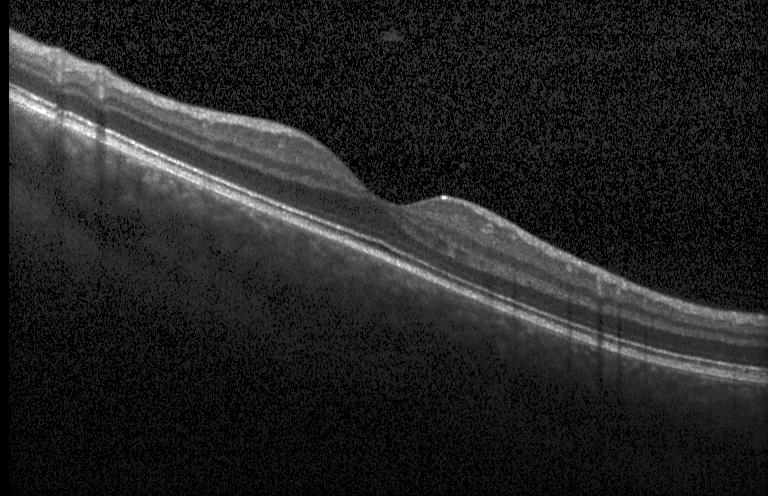
Horizontal scan through the fovea · retinal OCT B-scan · Heidelberg Spectralis · spectral-domain OCT — Assessment: no choroidal neovascularization, no diabetic macular edema, and no drusen.